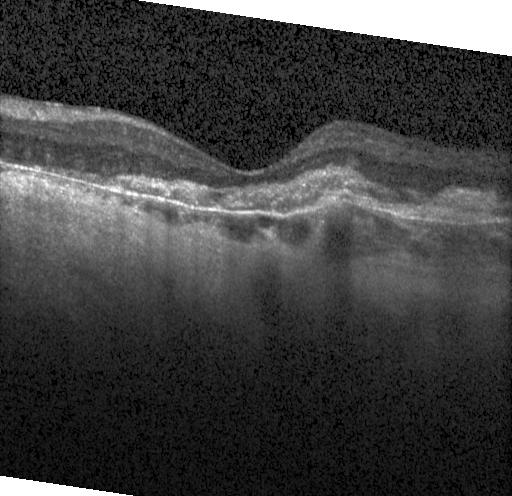
Optical coherence tomography B-scan — Finding: choroidal neovascularization (CNV).